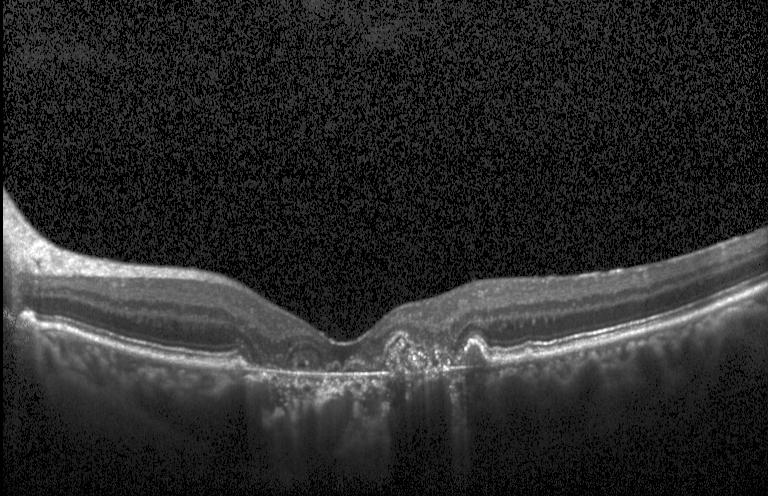
SD-OCT · retinal OCT cross-section · fovea-centered — This B-scan demonstrates choroidal neovascularization.